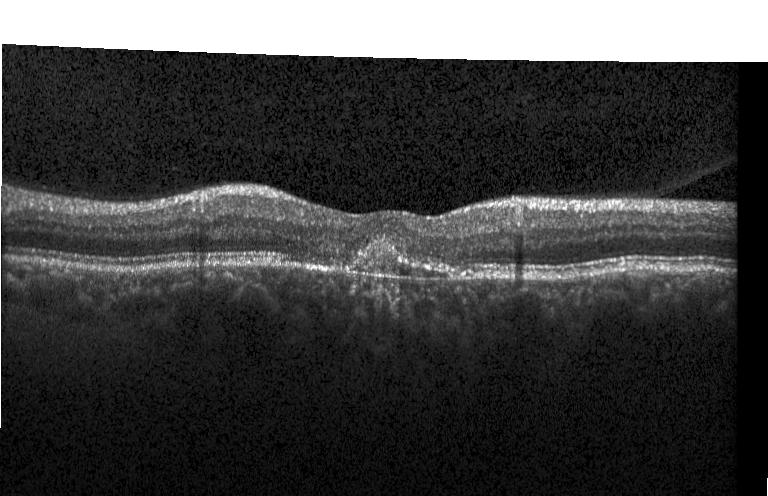

Retinal OCT cross-section, instrument: Heidelberg Spectralis.
Impression: a choroidal neovascular membrane.